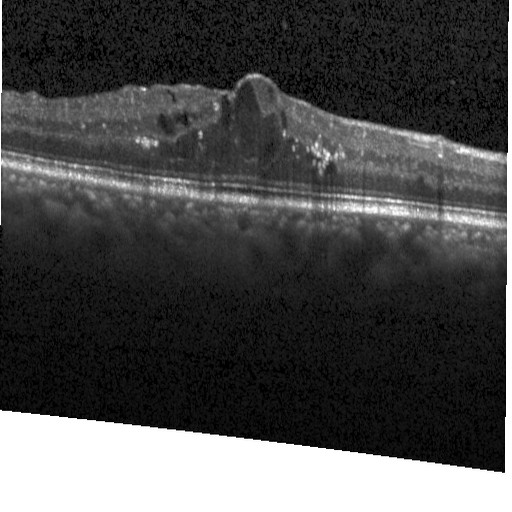 OCT finding: diabetic macular edema.